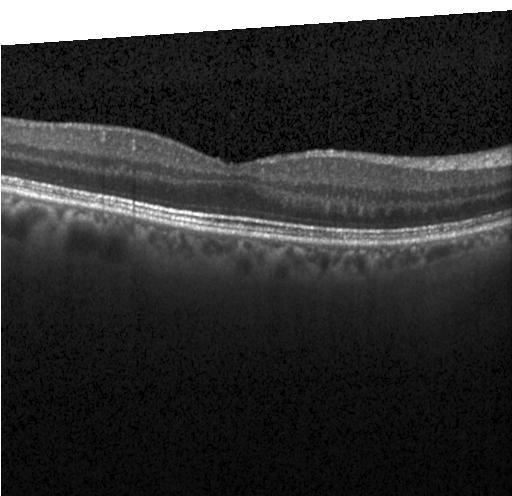

Finding: no evidence of choroidal neovascularization, diabetic macular edema, or drusen.